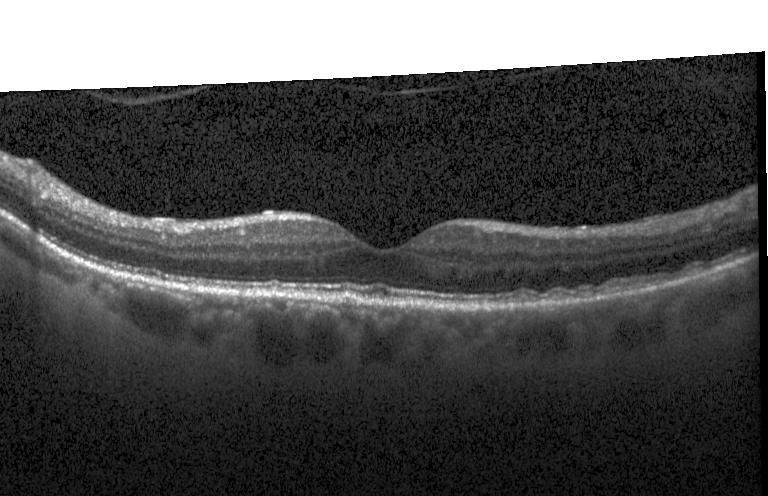
SD-OCT · OCT line scan. Diagnosis: multiple drusen.